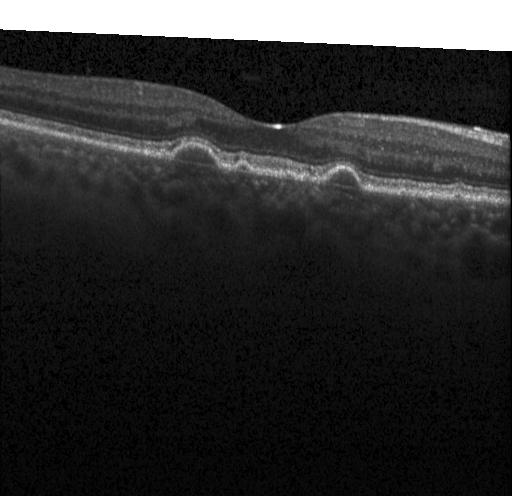

OCT line scan. Acquired on a Heidelberg Spectralis
Diagnosis: drusen.